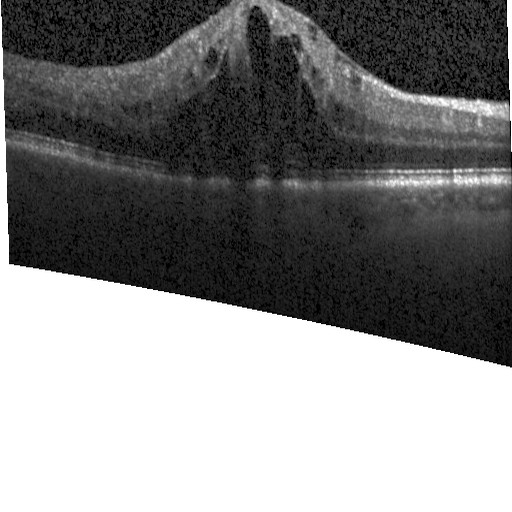
The scan shows diabetic macular edema (DME).